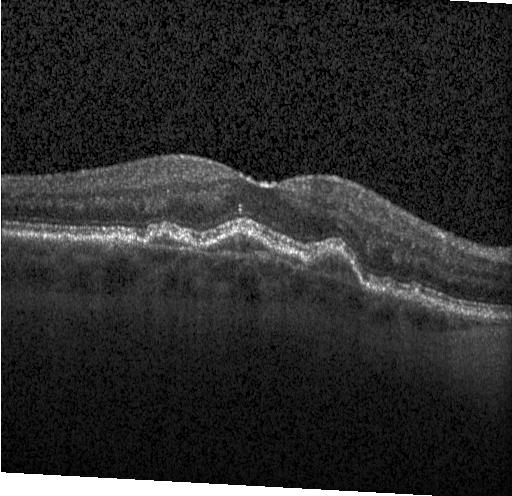
Spectral-domain OCT B-scan: choroidal neovascularization (CNV).